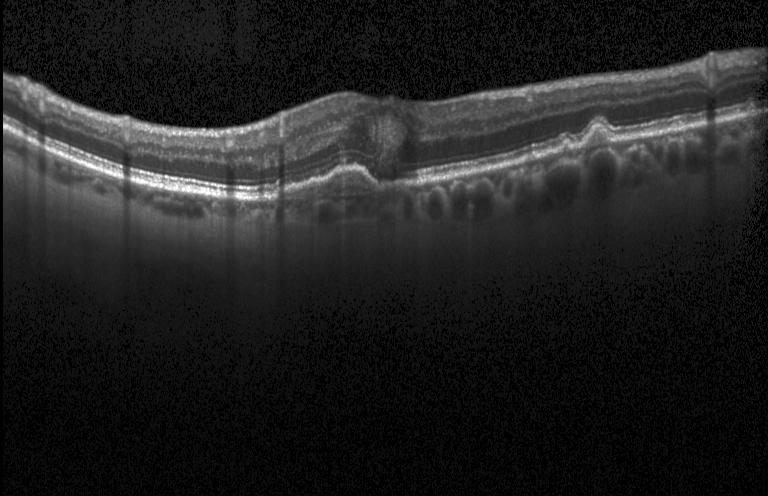

OCT B-scan showing CNV.